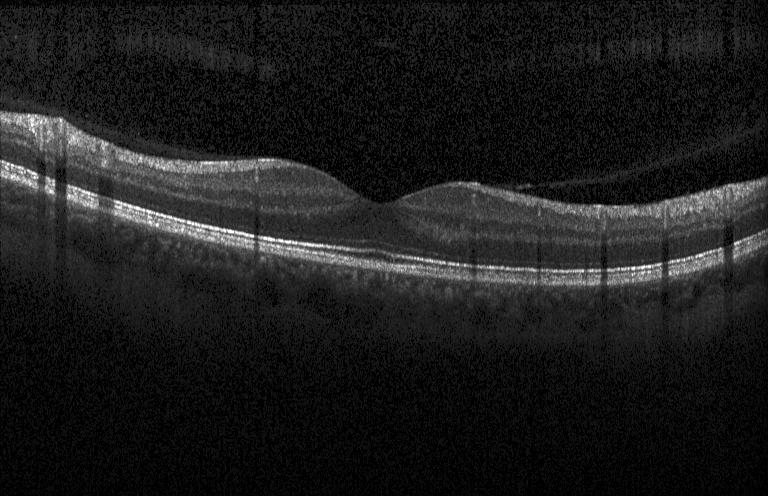 Horizontal scan through the fovea. OCT B-scan.
Dx: no evidence of CNV, DME, or drusen.